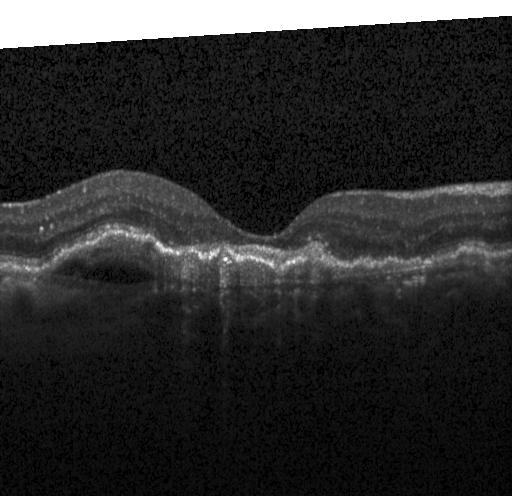 OCT B-scan
This B-scan demonstrates a choroidal neovascular membrane.